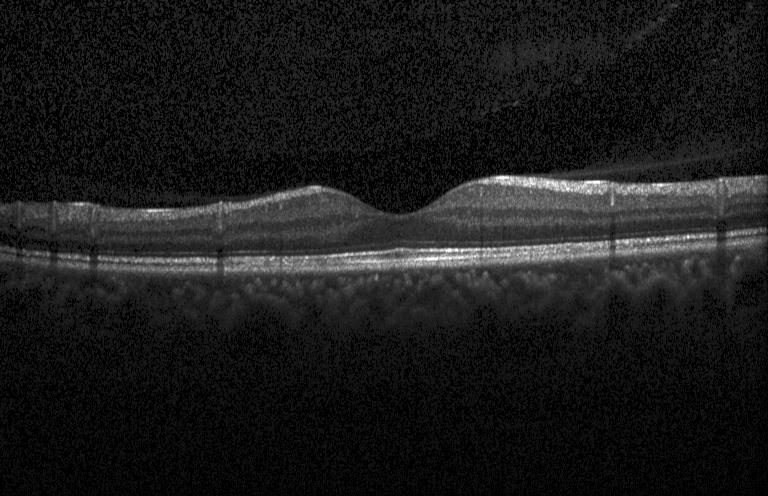

Impression: neither CNV, DME, nor drusen.